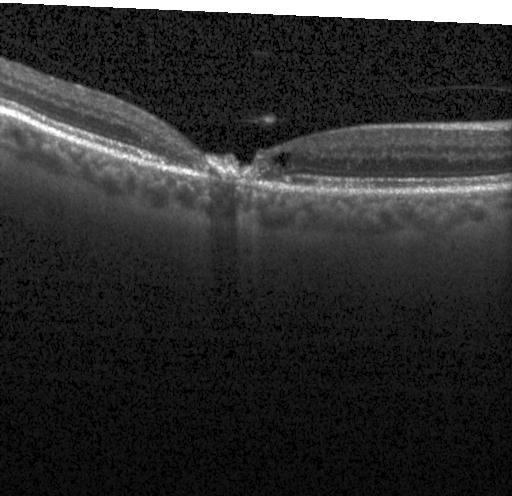

Macular OCT: CNV.